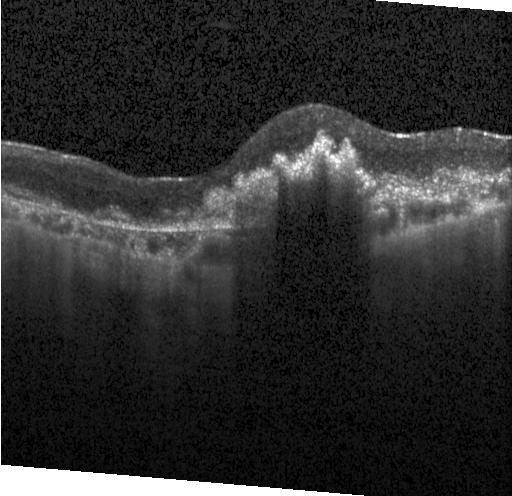
Macular OCT demonstrating a choroidal neovascular membrane.